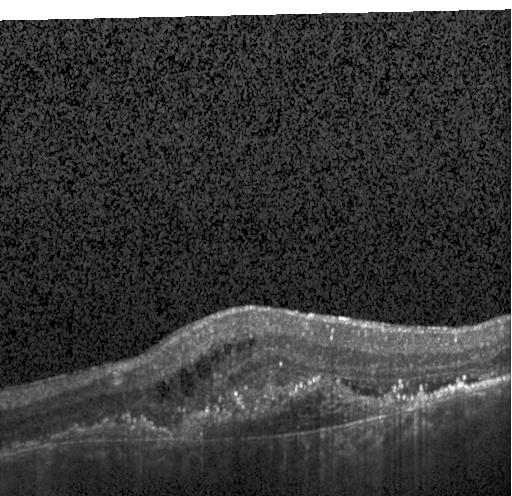
Spectral-domain optical coherence tomography; fovea-centered; acquired on a Heidelberg Spectralis; retinal OCT cross-section — Diagnosis: a choroidal neovascular membrane.